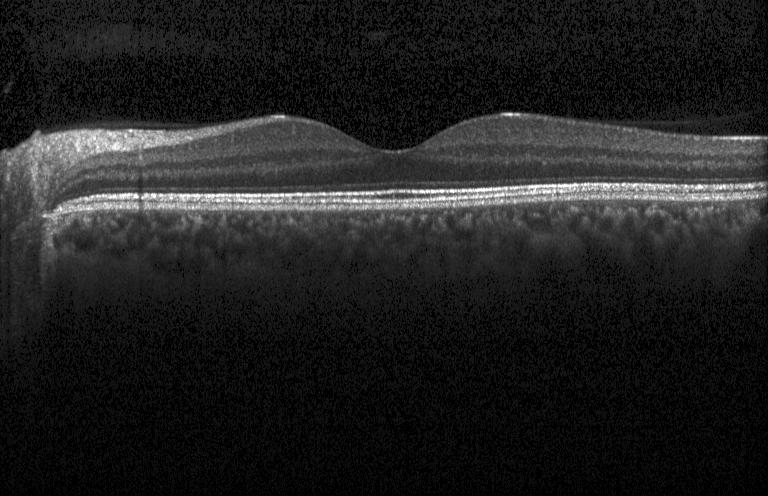 Impression: no evidence of choroidal neovascularization, diabetic macular edema, or drusen.